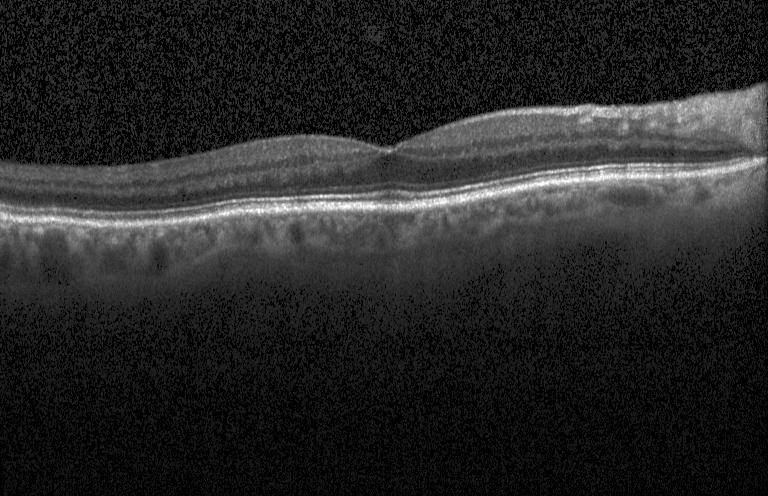
Macular OCT: neither choroidal neovascularization, diabetic macular edema, nor drusen.